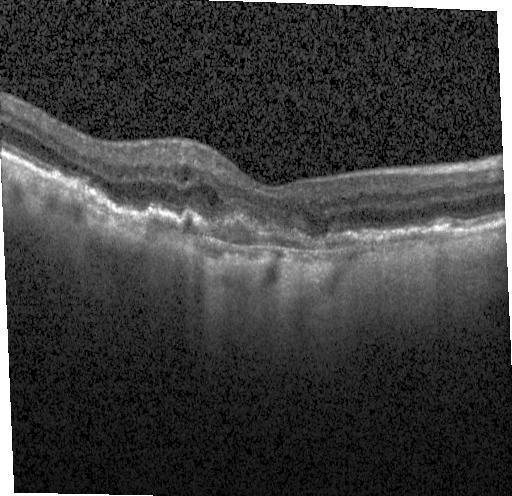 Acquired on a Heidelberg Spectralis. Centered on the fovea. OCT line scan — Dx: a choroidal neovascular membrane.